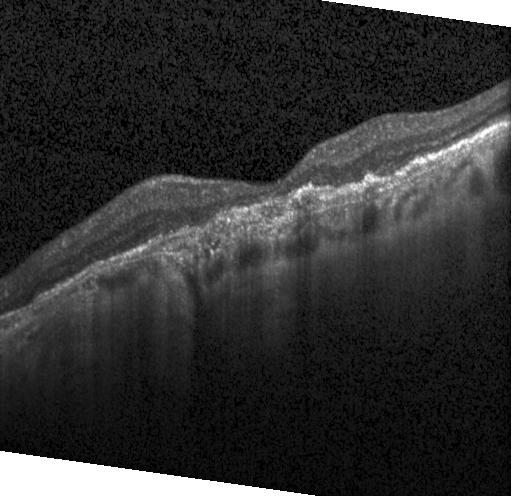

Retinal OCT B-scan · SD-OCT
Assessment: choroidal neovascularization.